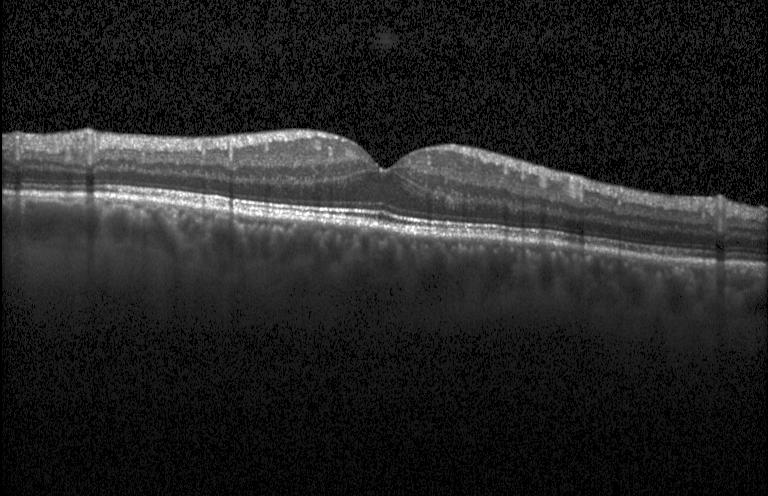 Finding: no CNV, no DME, and no drusen.